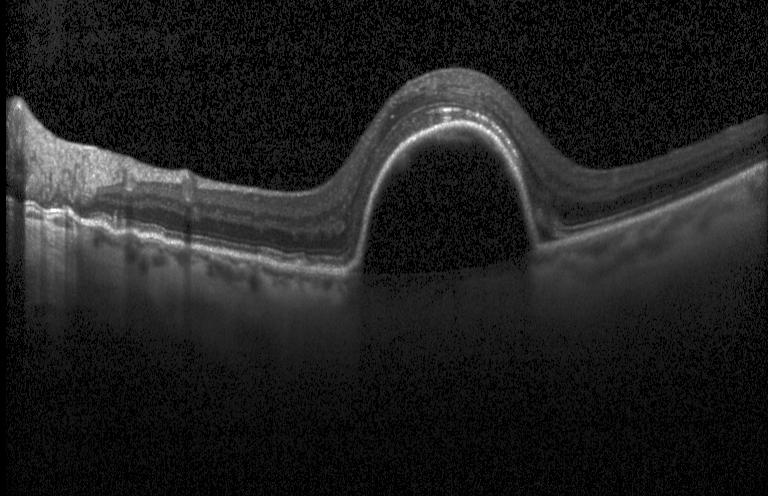

Spectral-domain OCT · OCT B-scan — Macular OCT: a choroidal neovascular membrane.